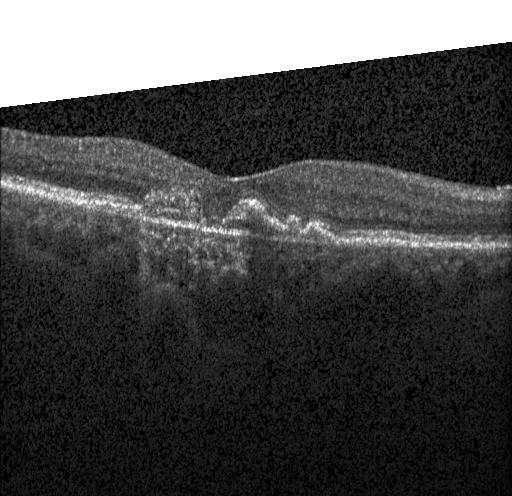
Acquired on a Heidelberg Spectralis · spectral-domain OCT · fovea-centered · optical coherence tomography scan.
Finding: a choroidal neovascular membrane.